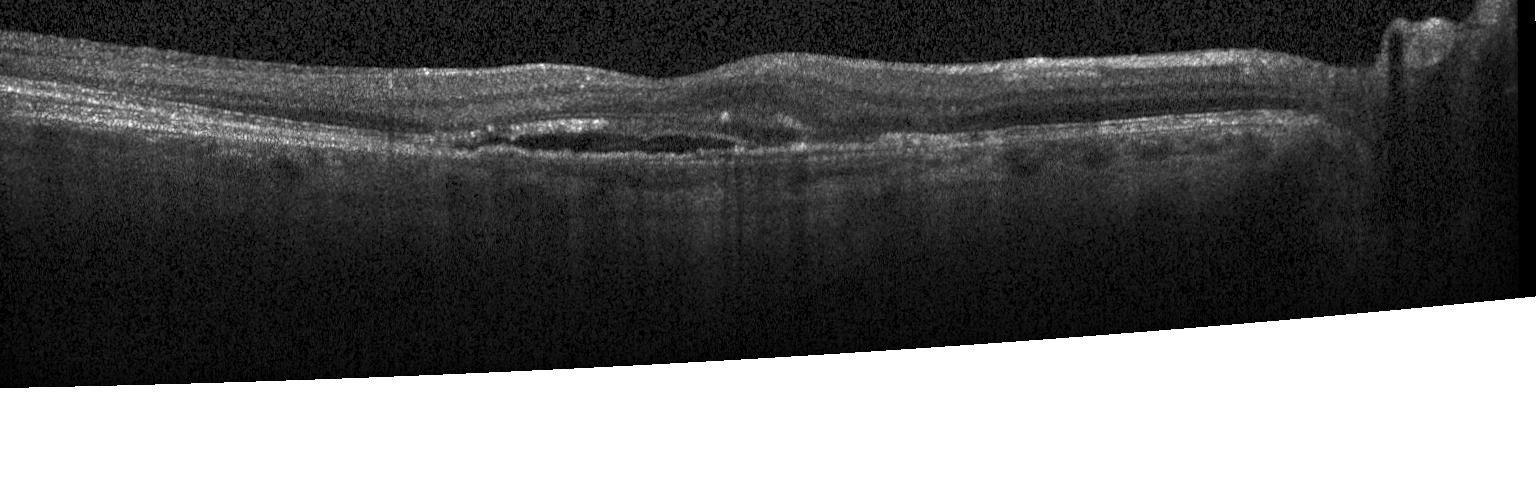

This B-scan demonstrates a choroidal neovascular membrane.